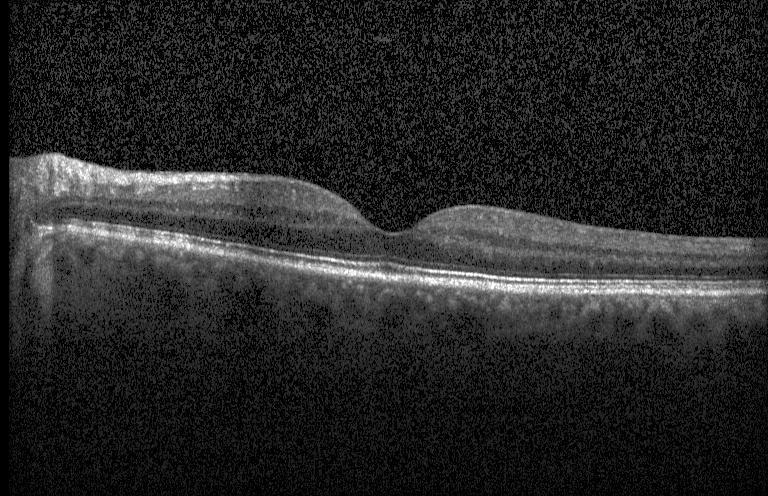

Centered on the fovea · retinal OCT B-scan. Finding: no evidence of CNV, DME, or drusen.